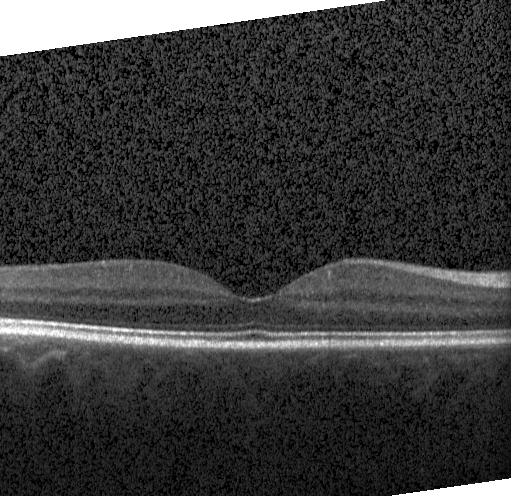 Centered on the fovea, optical coherence tomography B-scan. OCT finding: no choroidal neovascularization, no diabetic macular edema, and no drusen.